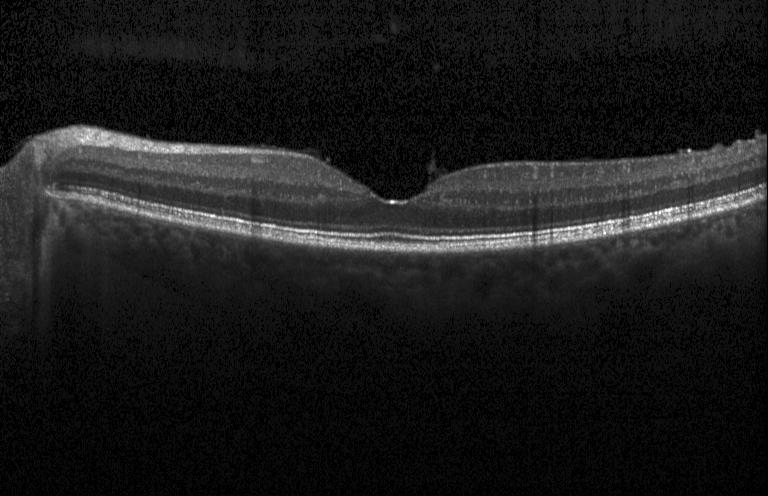
Optical coherence tomography B-scan.
Dx: no CNV, no DME, and no drusen.